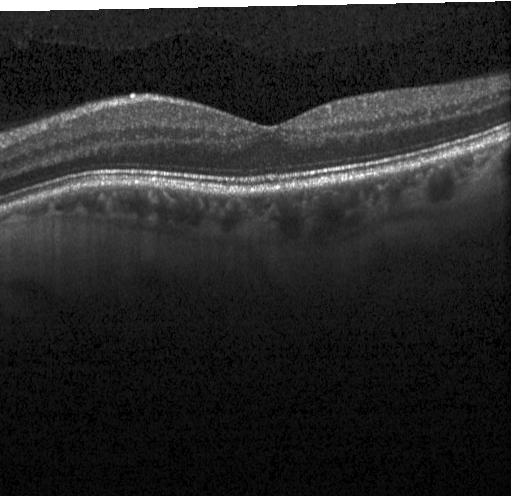
Diagnosis: no evidence of CNV, DME, or drusen.